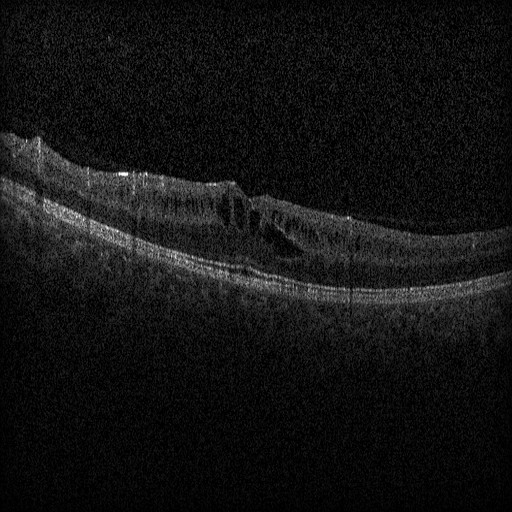 Optical coherence tomography scan, Heidelberg Spectralis OCT system
The scan shows diabetic macular edema.